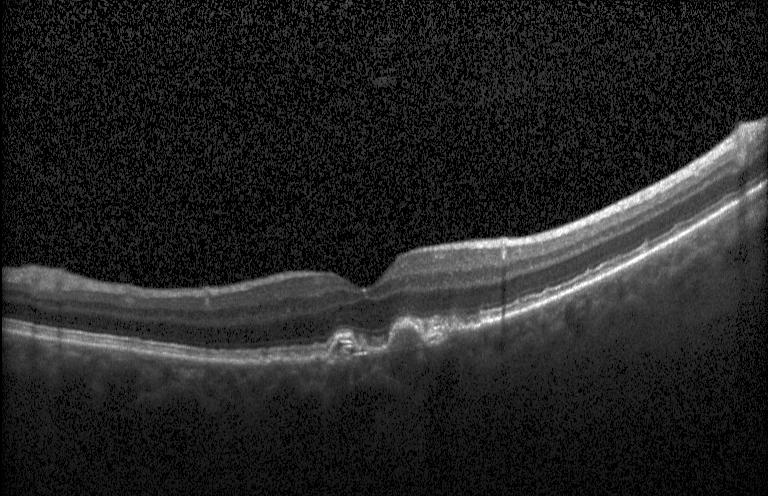 Retinal OCT cross-section showing choroidal neovascularization (CNV).